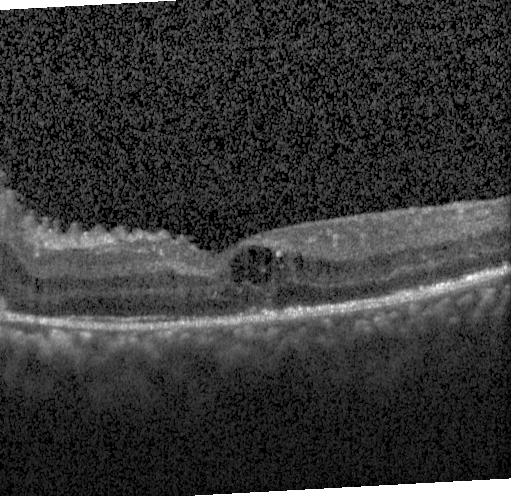
Diagnosis: DME.